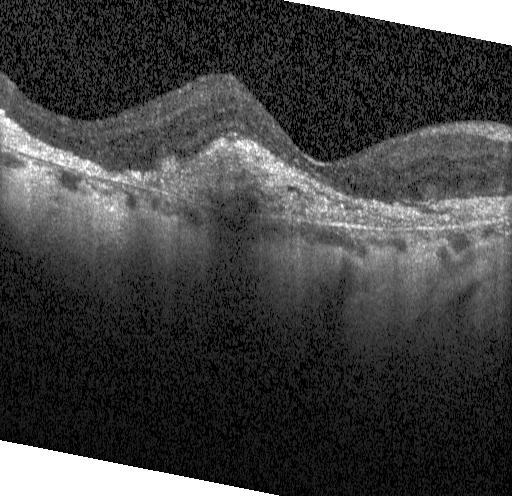

Optical coherence tomography scan, instrument: Heidelberg Spectralis.
This B-scan demonstrates choroidal neovascularization (CNV).